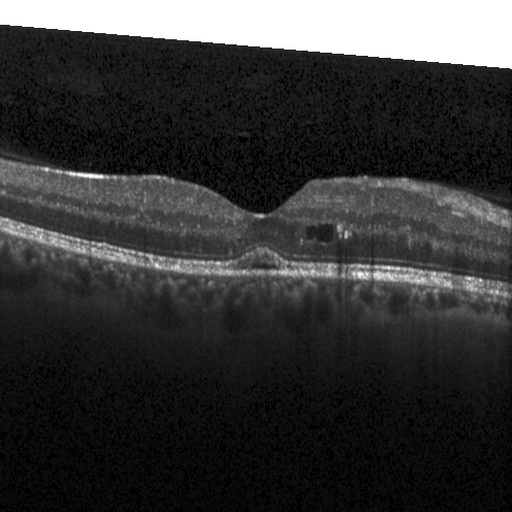 Horizontal scan through the fovea; Heidelberg Spectralis OCT system; retinal OCT cross-section; SD-OCT.
Impression: diabetic macular edema.